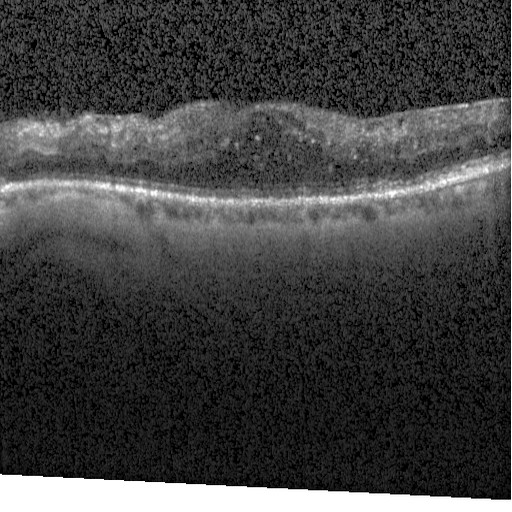 OCT finding: DME.